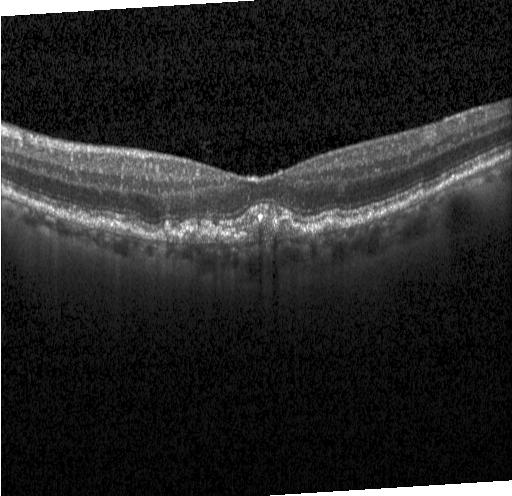 Retinal OCT cross-section; spectral-domain optical coherence tomography; acquired on a Heidelberg Spectralis; through the macula.
Diagnosis: sub-RPE drusenoid deposits.